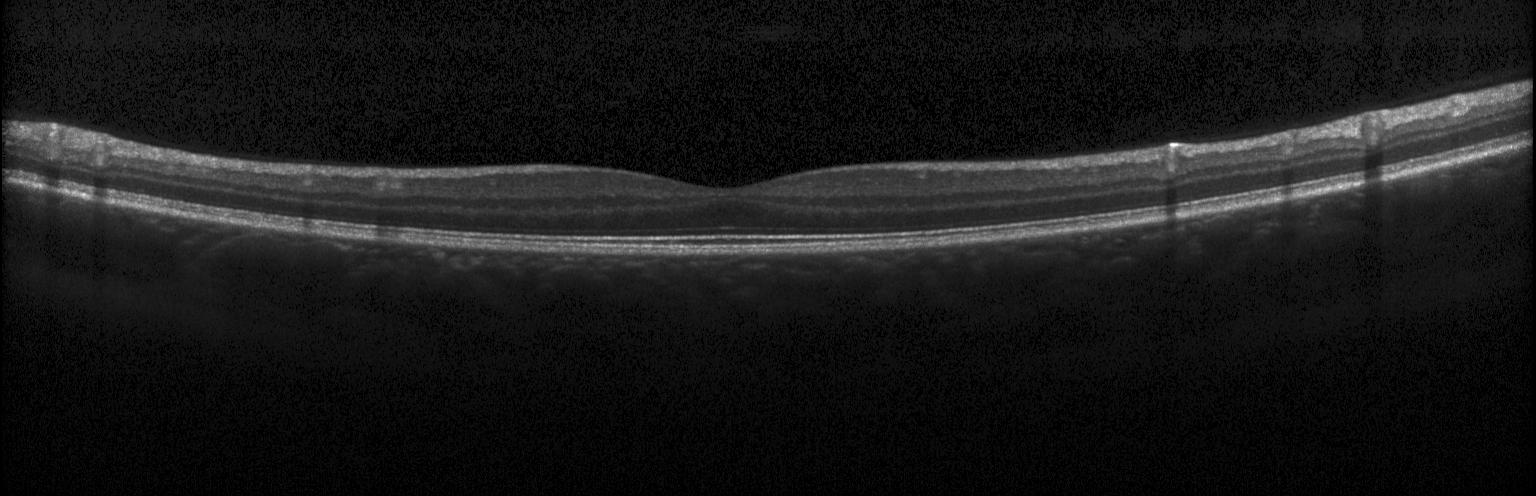 Horizontal scan through the fovea, optical coherence tomography B-scan, SD-OCT.
The scan shows no choroidal neovascularization, no diabetic macular edema, and no drusen.